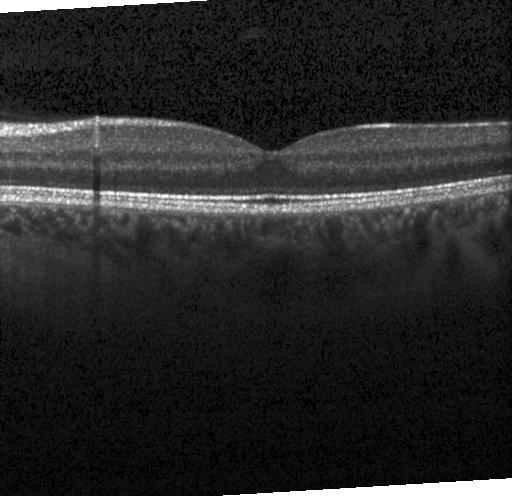 SD-OCT · optical coherence tomography B-scan · horizontal scan through the fovea · instrument: Heidelberg Spectralis
Macular OCT: no choroidal neovascularization, diabetic macular edema, or drusen.